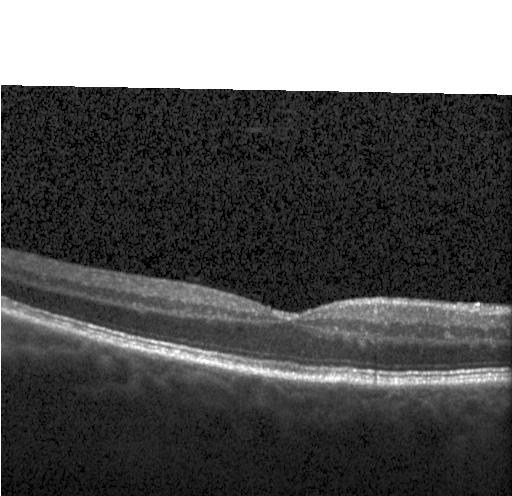

Impression: neither choroidal neovascularization, diabetic macular edema, nor drusen.